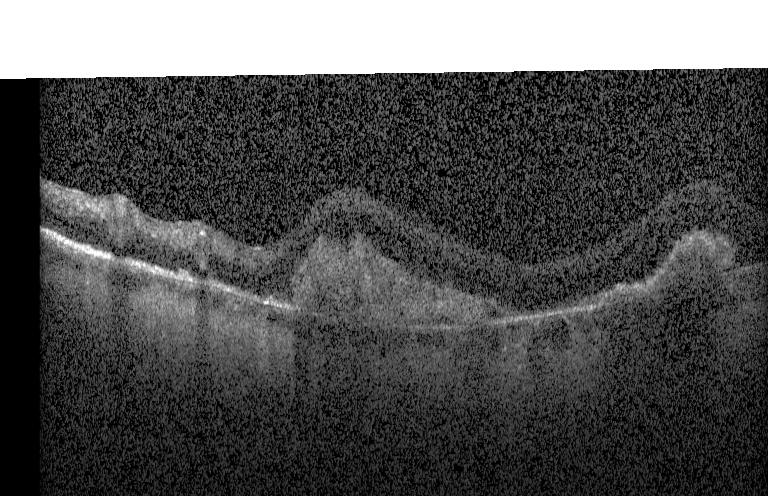
Fovea-centered, Heidelberg Spectralis OCT system, OCT B-scan. Dx: a choroidal neovascular membrane.